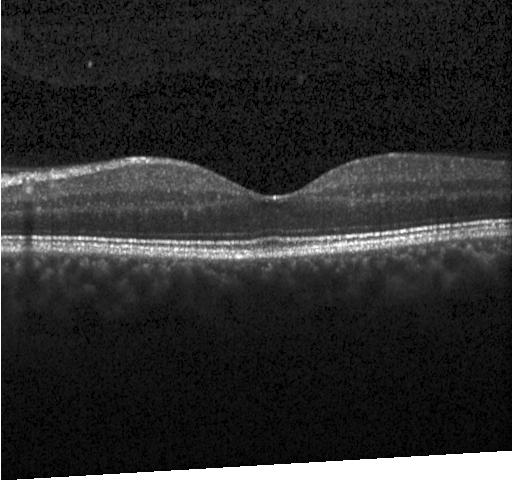
Optical coherence tomography B-scan. Dx: neither choroidal neovascularization, diabetic macular edema, nor drusen.